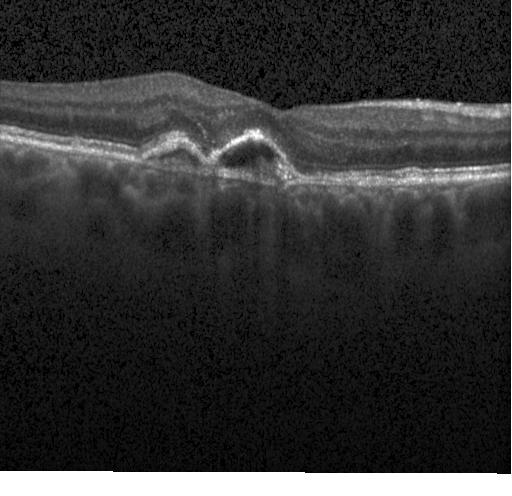 Macular OCT demonstrating choroidal neovascularization (CNV).